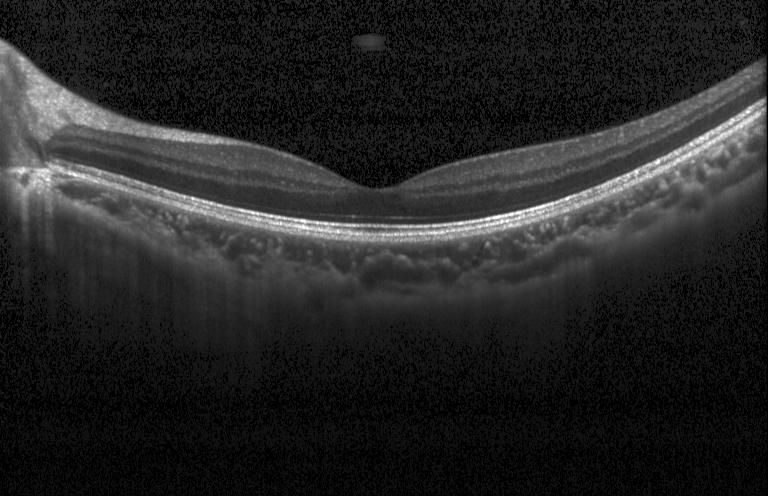 Heidelberg Spectralis OCT system · OCT B-scan · spectral-domain OCT. OCT finding: no evidence of CNV, DME, or drusen.